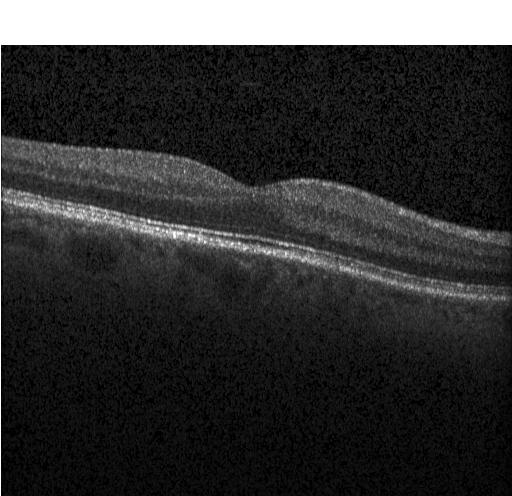 OCT B-scan.
Impression: no CNV, no DME, and no drusen.